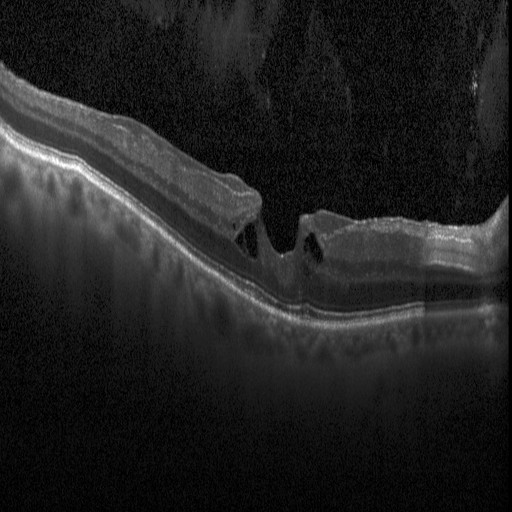
Optical coherence tomography scan — Finding: DME.